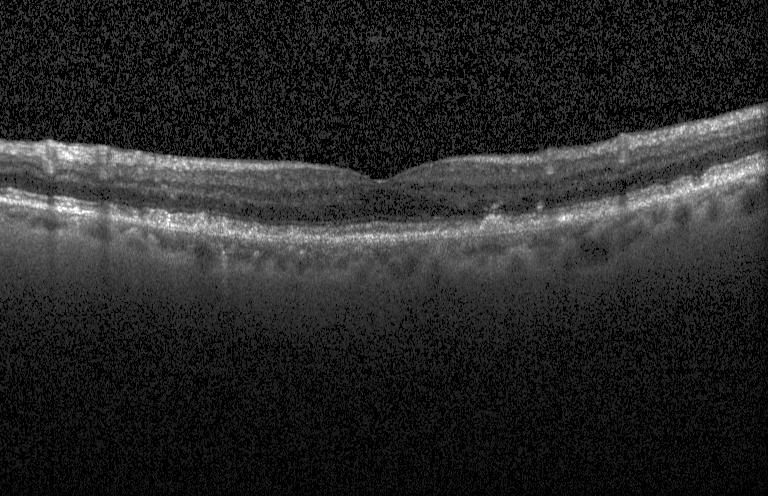 Assessment: sub-RPE drusenoid deposits.